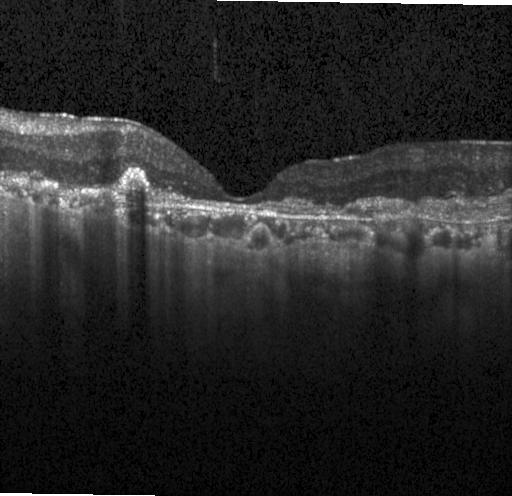
Diagnosis: choroidal neovascularization (CNV).